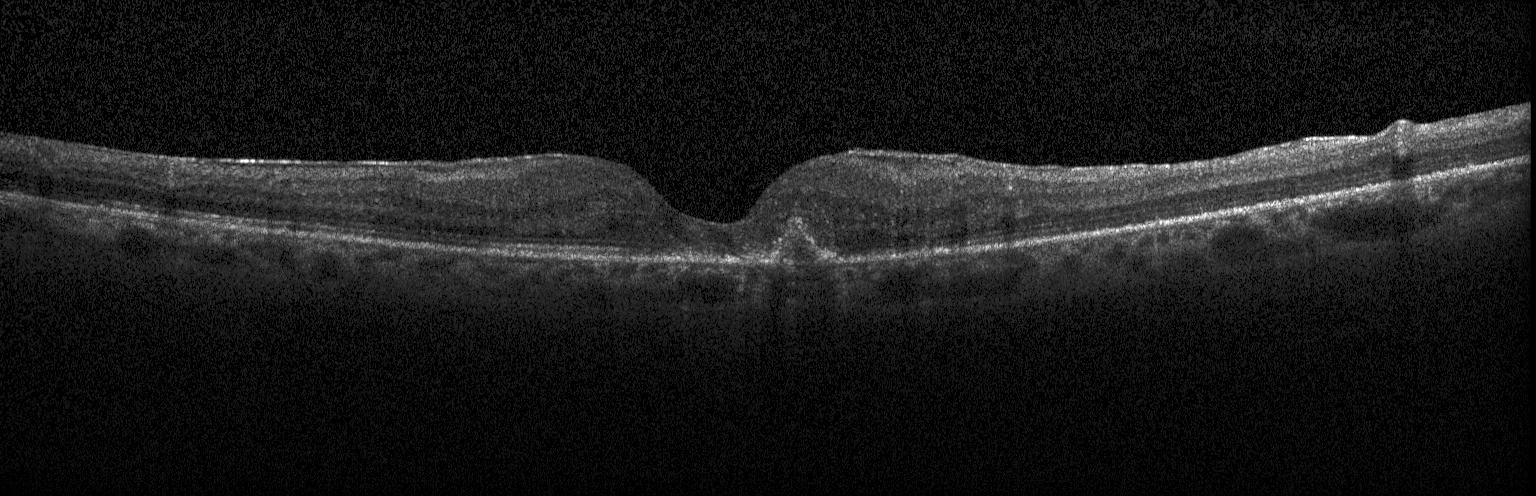

Retinal OCT cross-section showing a choroidal neovascular membrane.